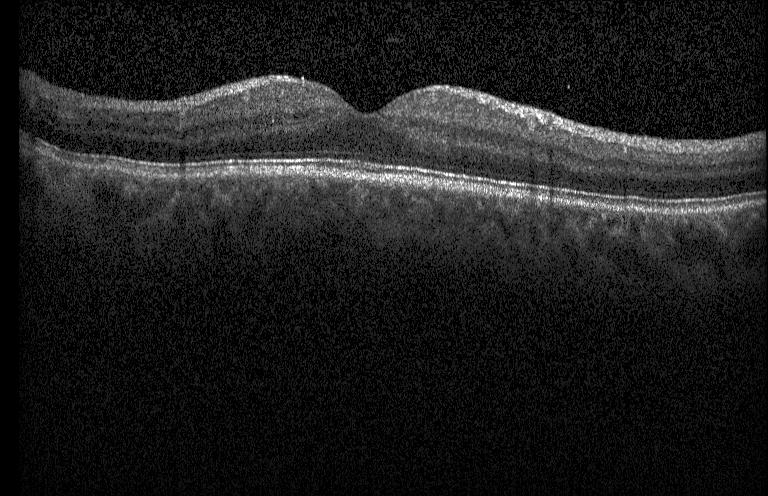
Spectral-domain OCT. Retinal OCT cross-section. Horizontal scan through the fovea.
Impression: neither choroidal neovascularization, diabetic macular edema, nor drusen.